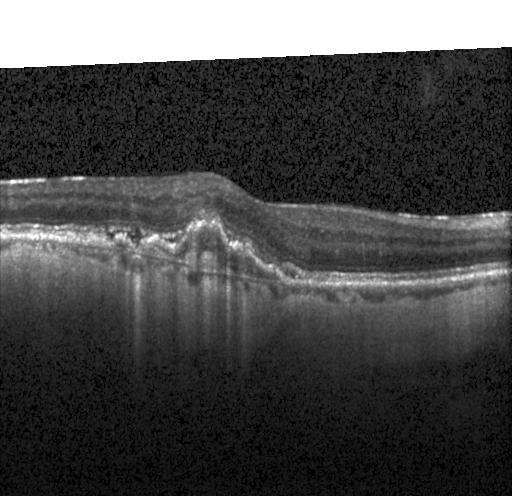

Optical coherence tomography scan. OCT finding: a choroidal neovascular membrane.